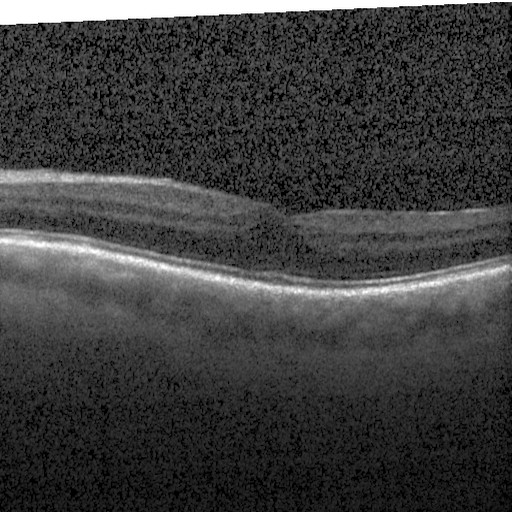 Assessment: DME.